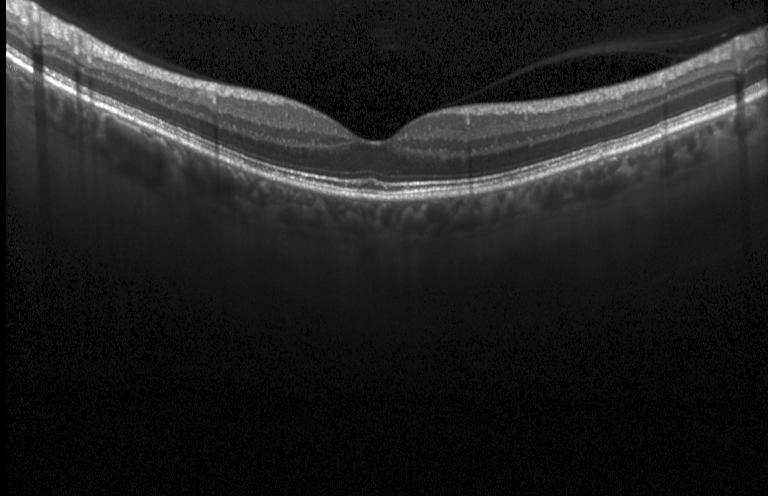

Macular OCT: no CNV, no DME, and no drusen.